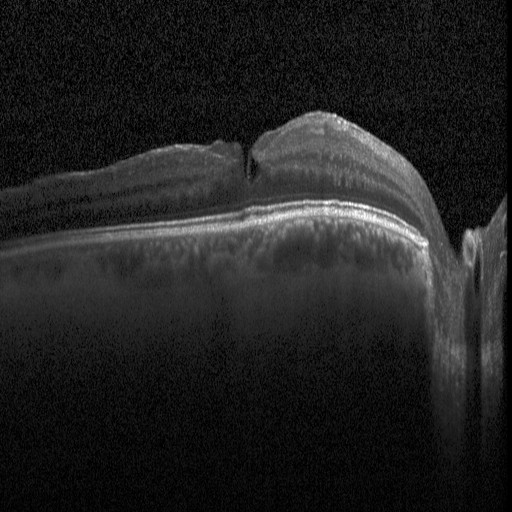
Optical coherence tomography scan
Assessment: diabetic macular edema.